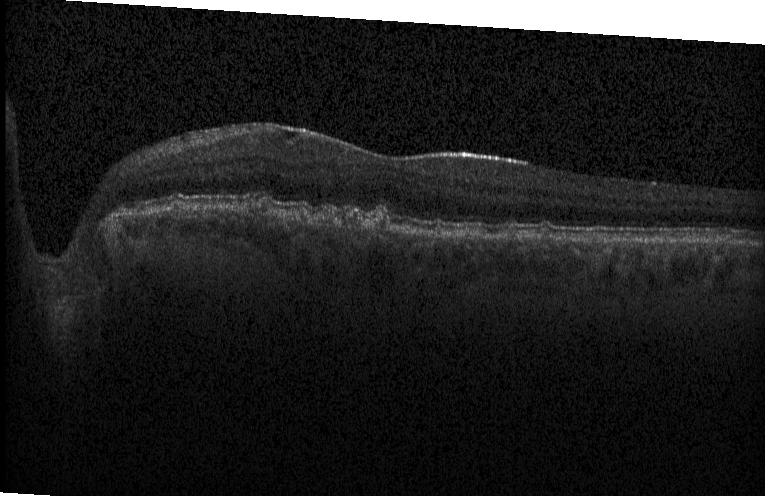

OCT B-scan.
Assessment: drusen.